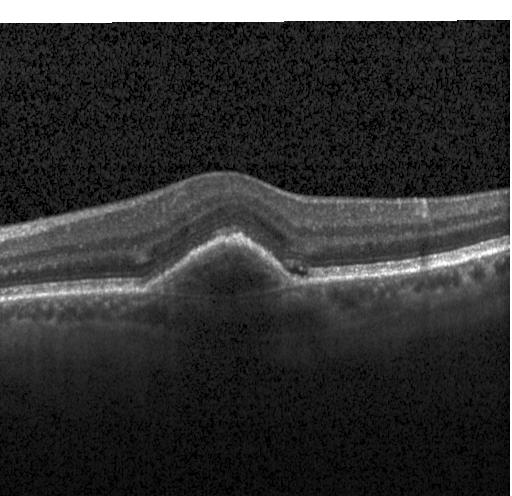

Optical coherence tomography B-scan; acquired on a Heidelberg Spectralis; SD-OCT — This B-scan demonstrates a choroidal neovascular membrane.